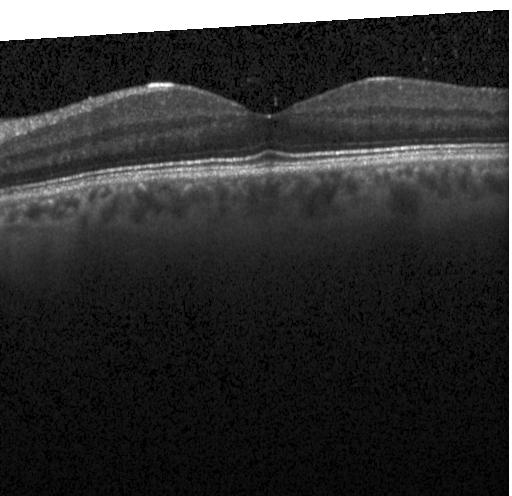 Optical coherence tomography scan. The scan shows no choroidal neovascularization, no diabetic macular edema, and no drusen.